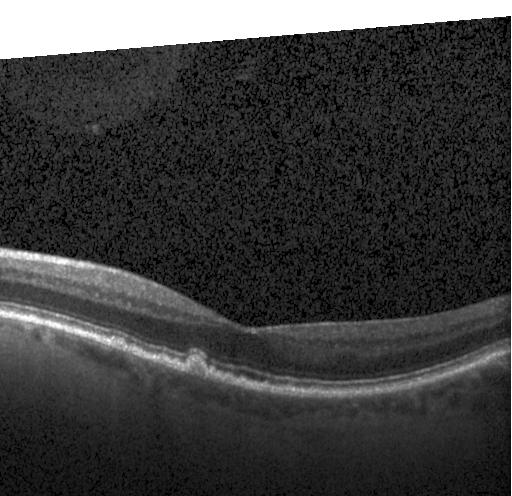 Diagnosis: multiple drusen.